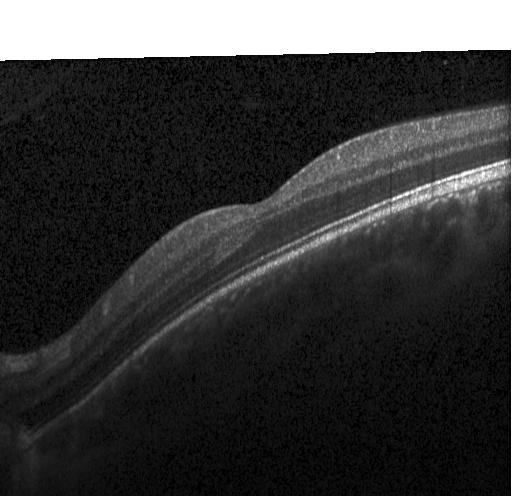
This B-scan demonstrates no CNV, DME, or drusen.